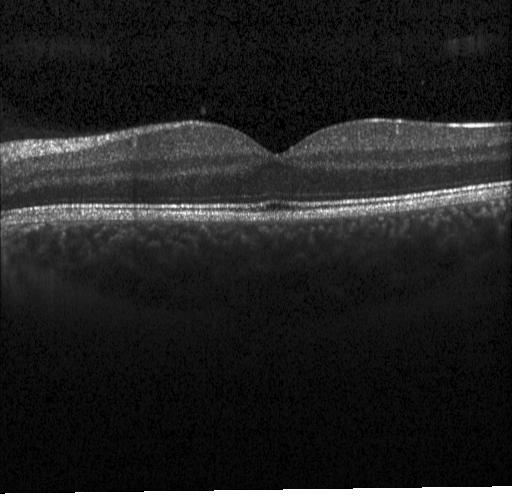

Optical coherence tomography B-scan. SD-OCT. Acquired on a Heidelberg Spectralis.
Assessment: no evidence of choroidal neovascularization, diabetic macular edema, or drusen.